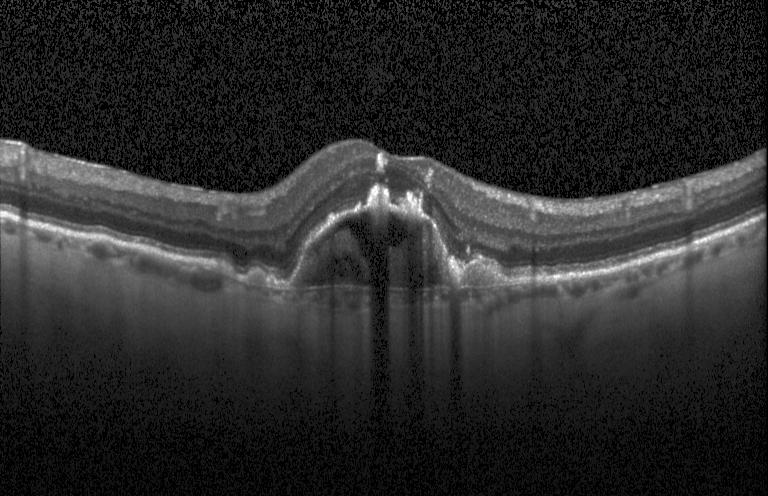

OCT B-scan. Heidelberg Spectralis. Horizontal scan through the fovea — Assessment: a choroidal neovascular membrane.